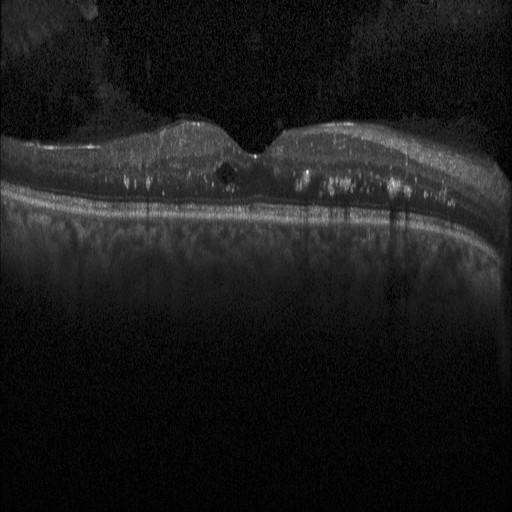

Dx: diabetic macular edema.